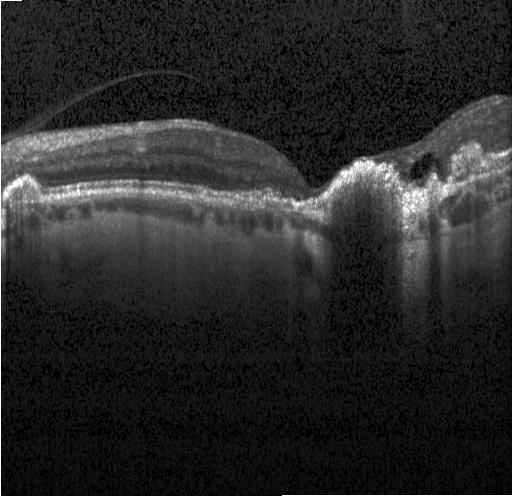

Choroidal neovascularization.